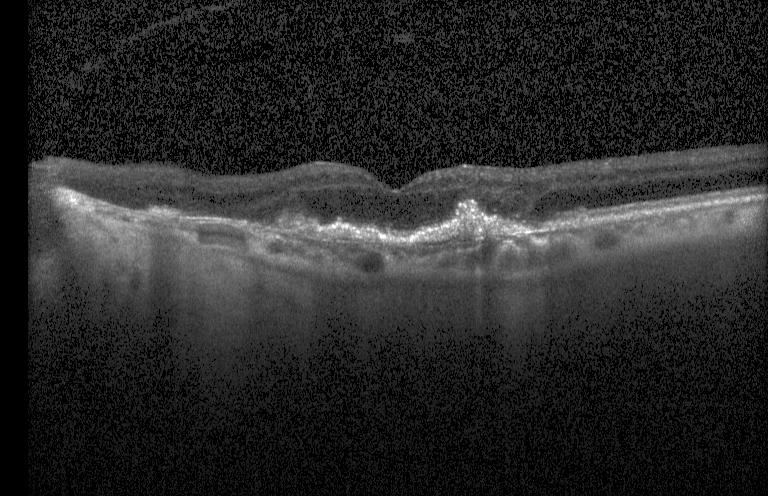
Horizontal scan through the fovea, retinal OCT B-scan, spectral-domain optical coherence tomography. Diagnosis: a choroidal neovascular membrane.